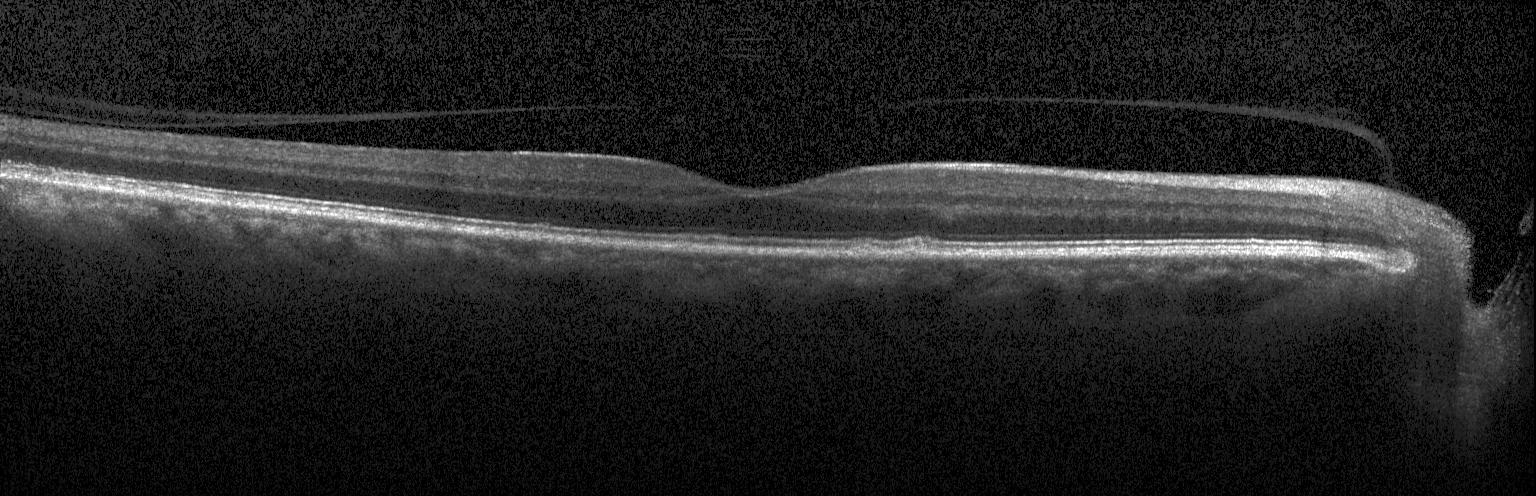
Assessment: sub-RPE drusenoid deposits.